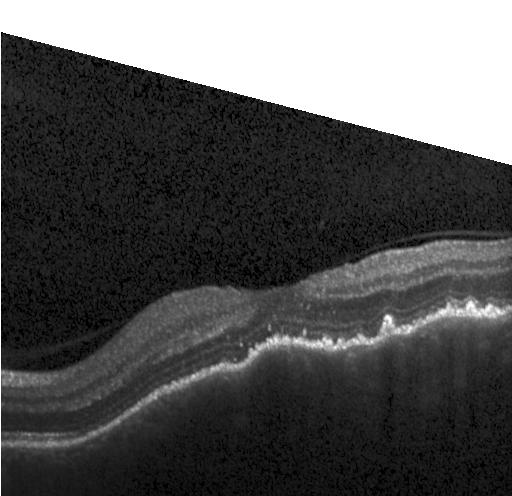 SD-OCT · OCT B-scan.
Diagnosis: sub-RPE drusenoid deposits.